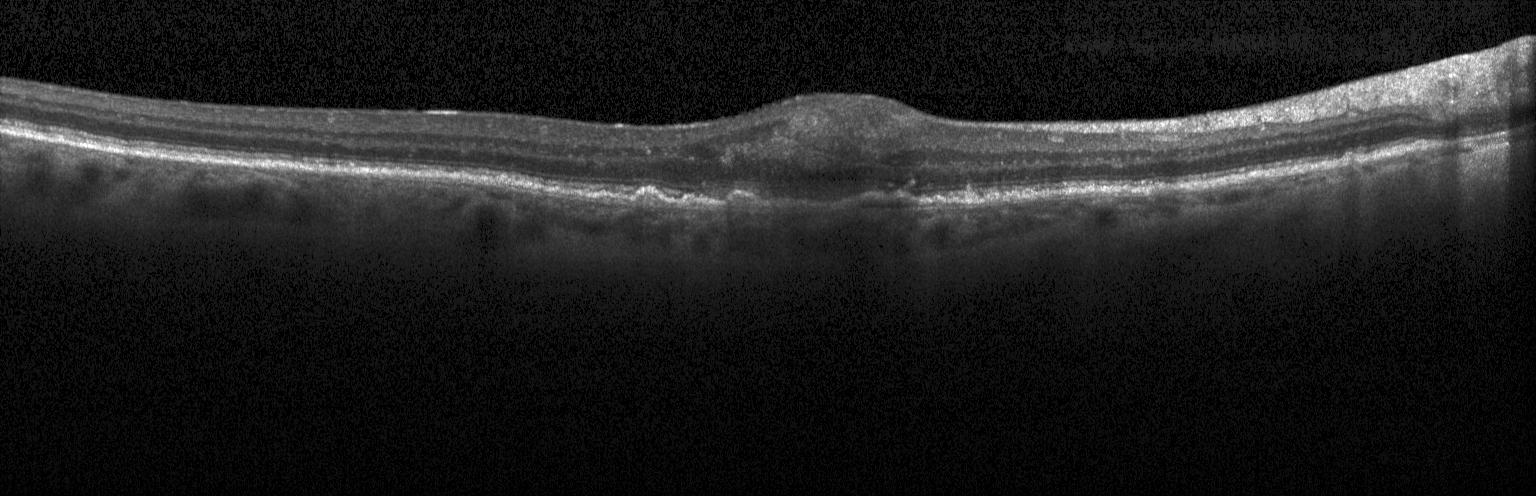

Impression: CNV.